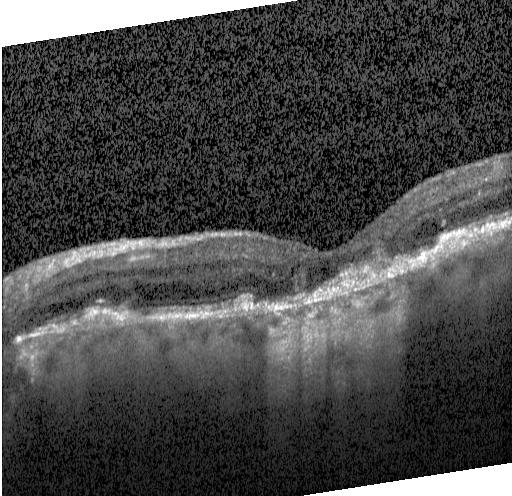

Spectral-domain OCT B-scan: a choroidal neovascular membrane.